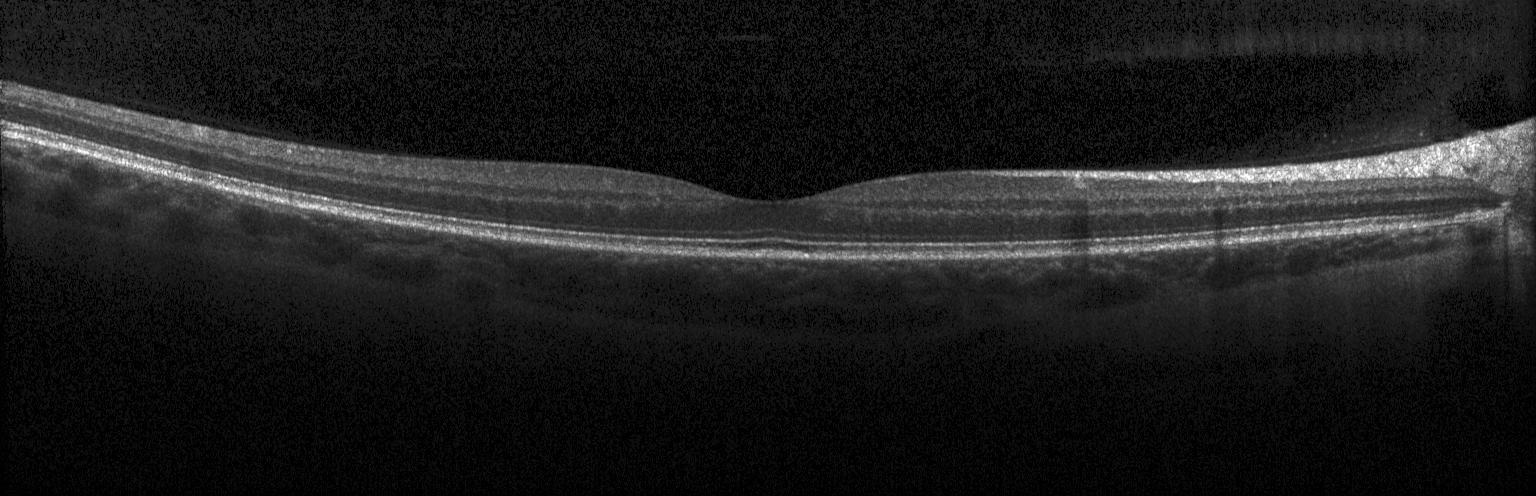

OCT B-scan. Assessment: neither CNV, DME, nor drusen.